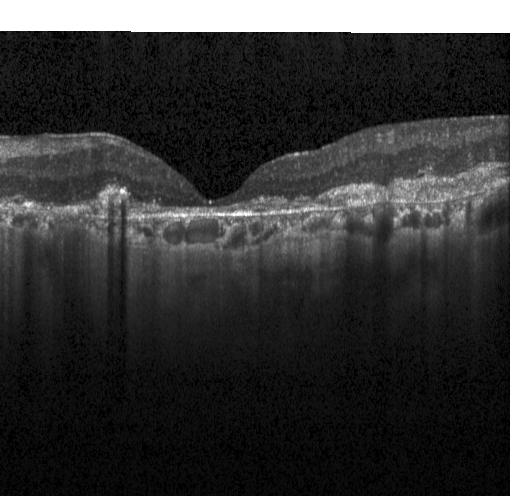

Retinal OCT B-scan. SD-OCT. Horizontal scan through the fovea.
Impression: a choroidal neovascular membrane.